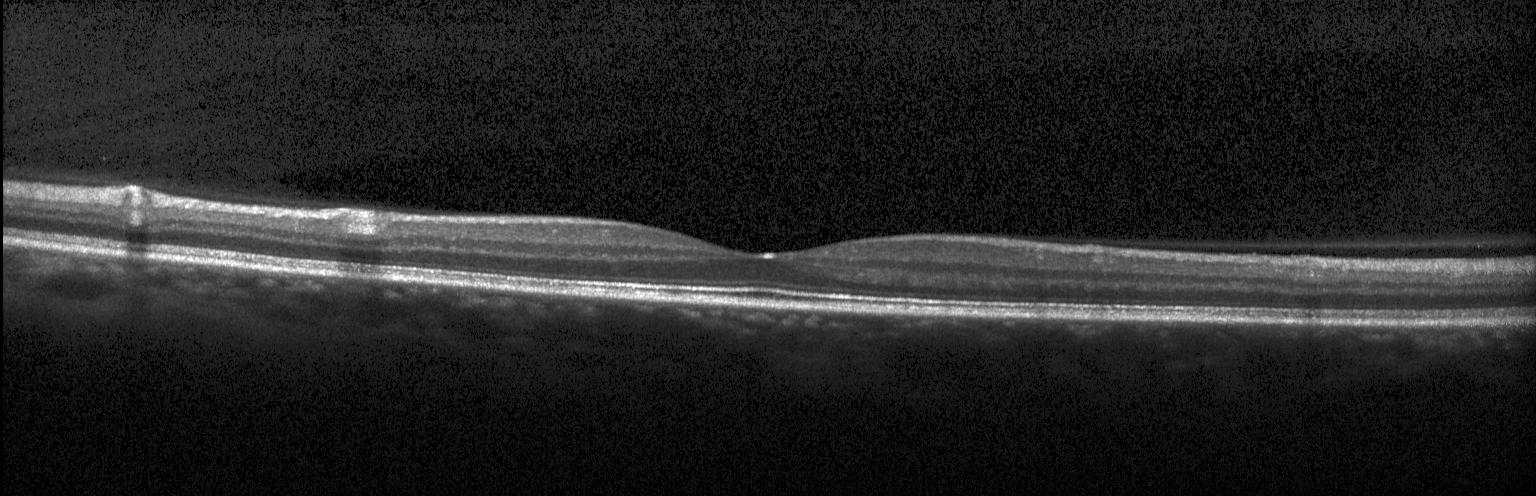

OCT B-scan · SD-OCT — The scan shows no evidence of CNV, DME, or drusen.